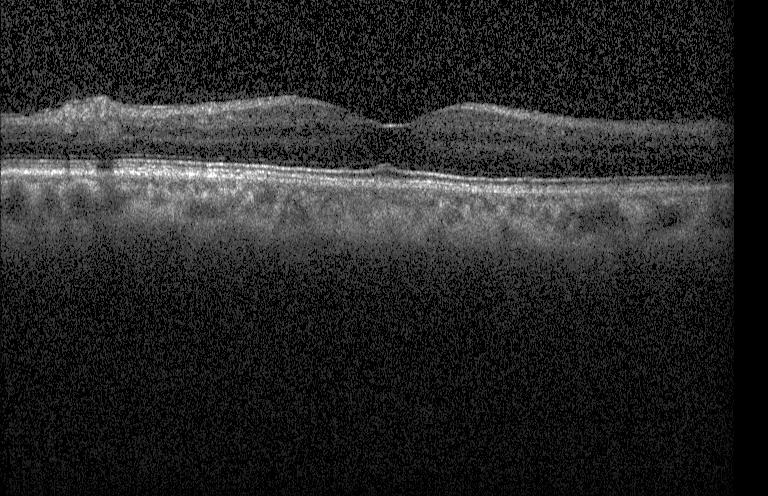 Spectral-domain optical coherence tomography; retinal OCT B-scan; horizontal scan through the fovea — Impression: neither CNV, DME, nor drusen.